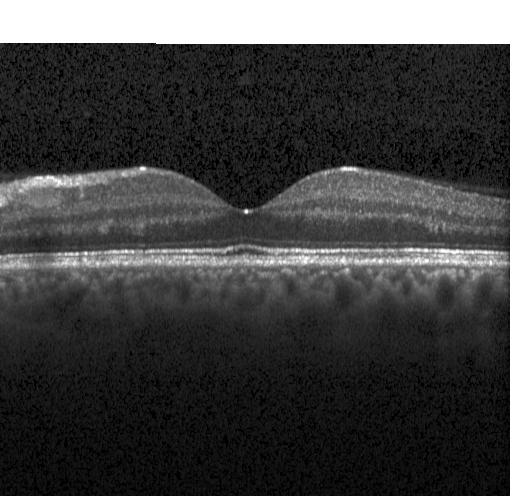
Retinal OCT cross-section showing no choroidal neovascularization, diabetic macular edema, or drusen.